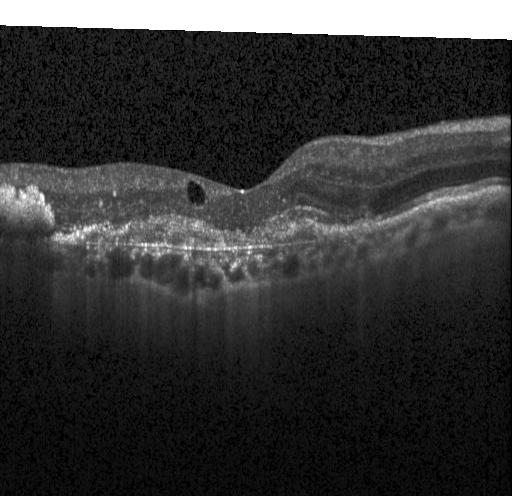 Heidelberg Spectralis, horizontal scan through the fovea, retinal OCT B-scan — Diagnosis: a choroidal neovascular membrane.